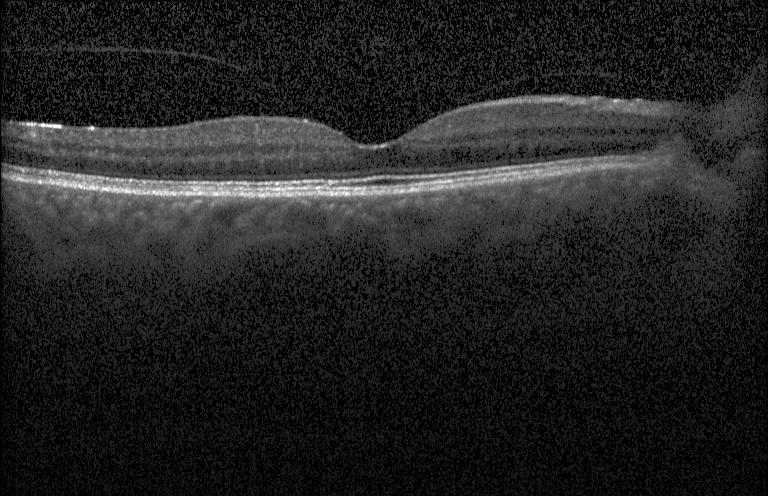

OCT scan showing no choroidal neovascularization, no diabetic macular edema, and no drusen.